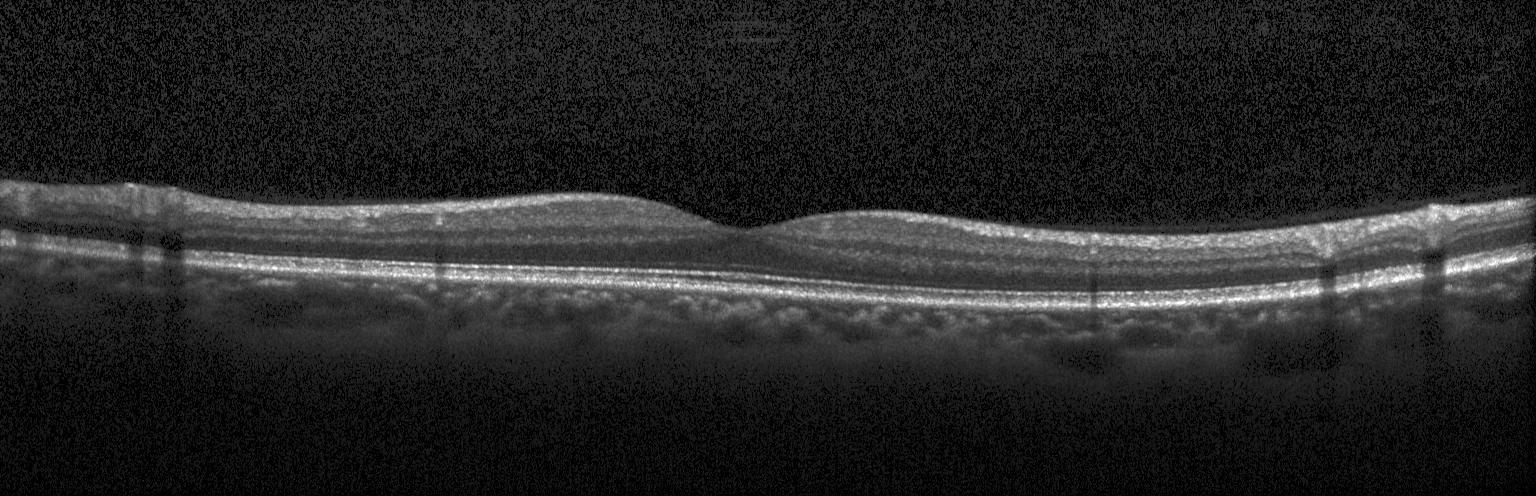 Spectral-domain OCT B-scan: no evidence of choroidal neovascularization, diabetic macular edema, or drusen.